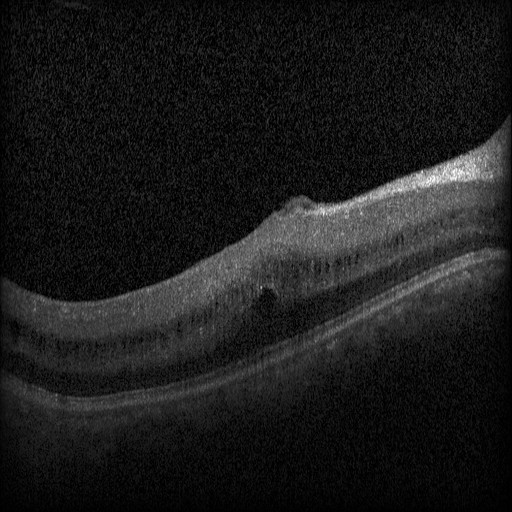 Impression: diabetic macular edema (DME).